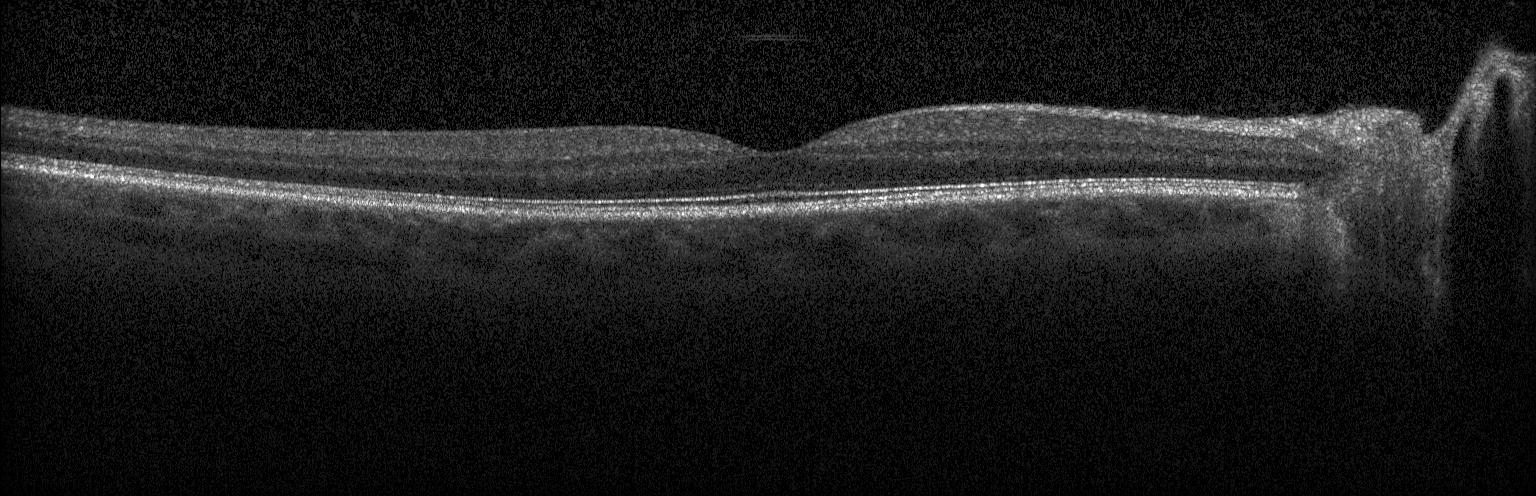
Retinal OCT B-scan. OCT finding: no choroidal neovascularization, diabetic macular edema, or drusen.